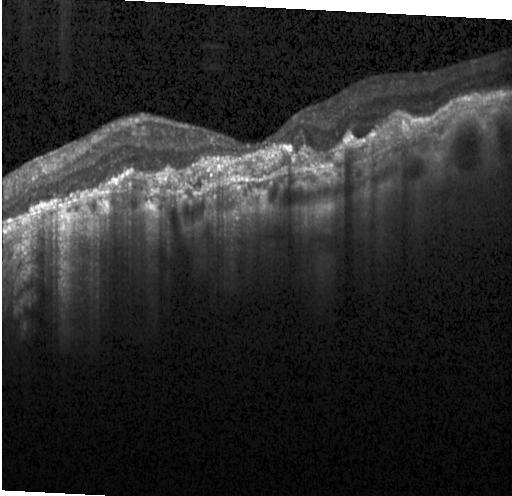 This B-scan demonstrates choroidal neovascularization (CNV).